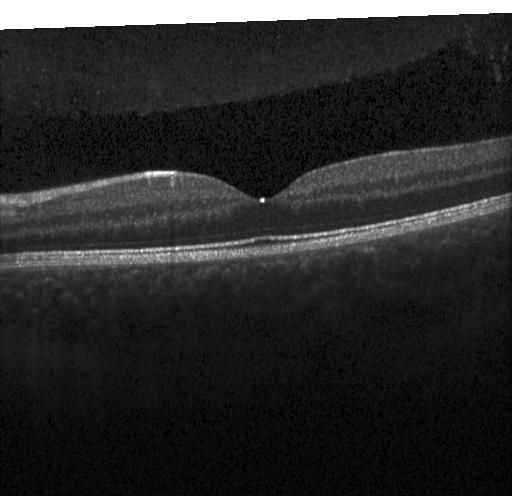

Retinal OCT cross-section
The scan shows no choroidal neovascularization, no diabetic macular edema, and no drusen.